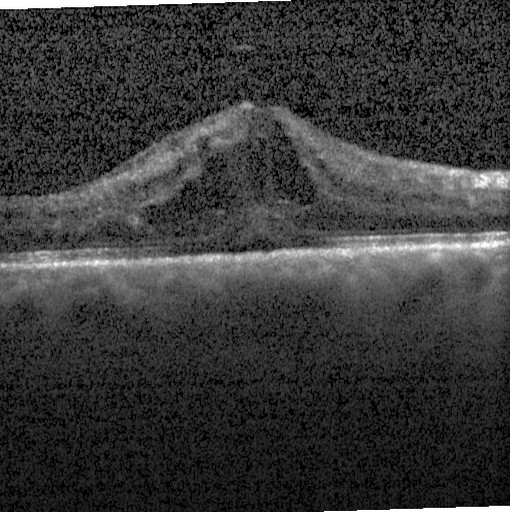 Diagnosis: diabetic macular edema (DME).